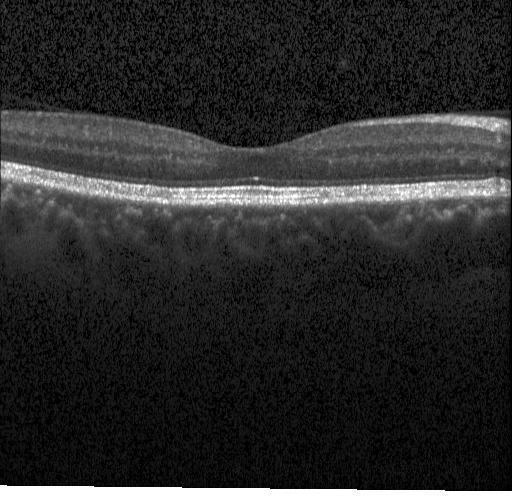 Macular OCT: no evidence of choroidal neovascularization, diabetic macular edema, or drusen.